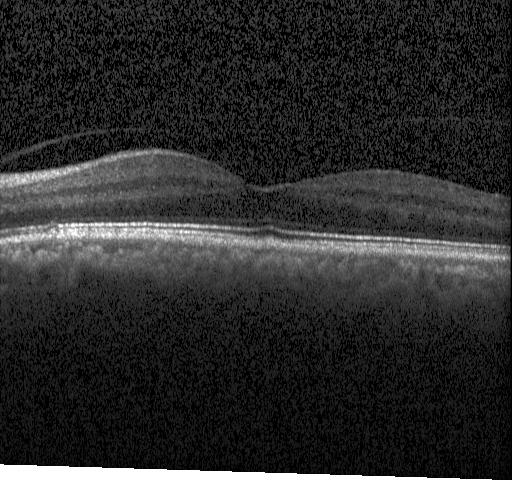 OCT B-scan, SD-OCT, instrument: Heidelberg Spectralis
Diagnosis: no choroidal neovascularization, diabetic macular edema, or drusen.